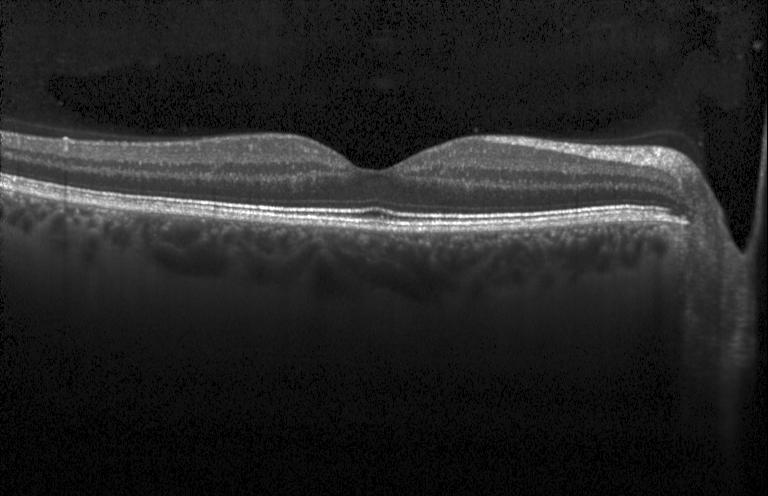

Dx: neither choroidal neovascularization, diabetic macular edema, nor drusen.